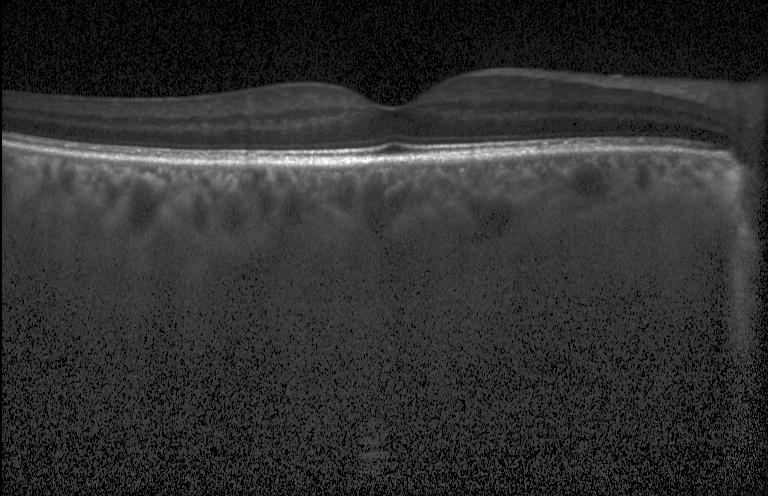

SD-OCT, macular scan, Heidelberg Spectralis OCT system, retinal OCT cross-section. Finding: neither choroidal neovascularization, diabetic macular edema, nor drusen.